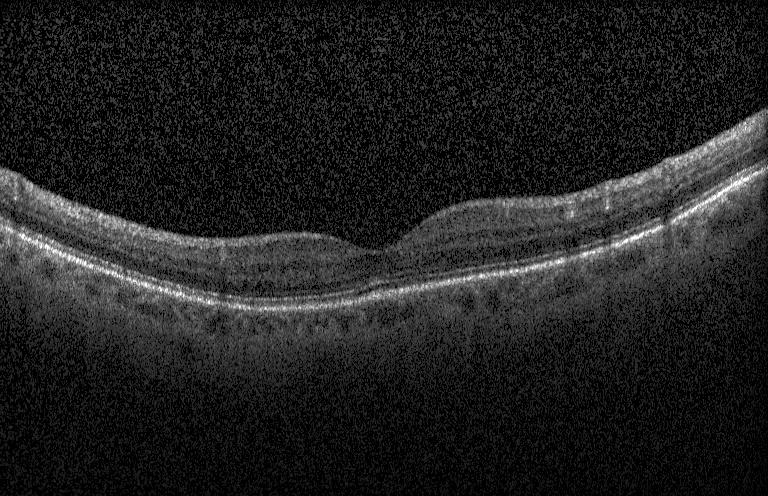 Spectral-domain optical coherence tomography; fovea-centered; acquired on a Heidelberg Spectralis; retinal OCT B-scan.
No choroidal neovascularization, diabetic macular edema, or drusen.